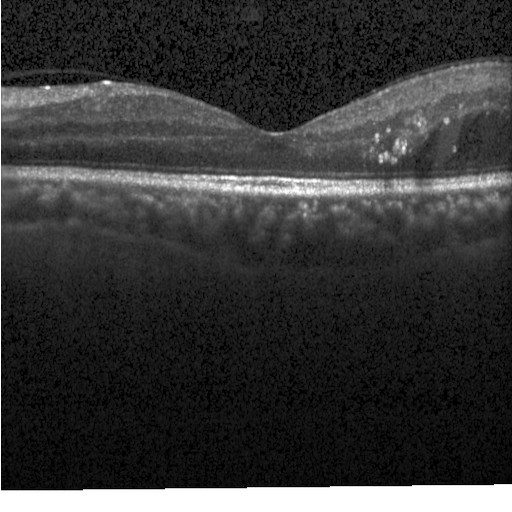

Macular OCT demonstrating diabetic macular edema (DME).